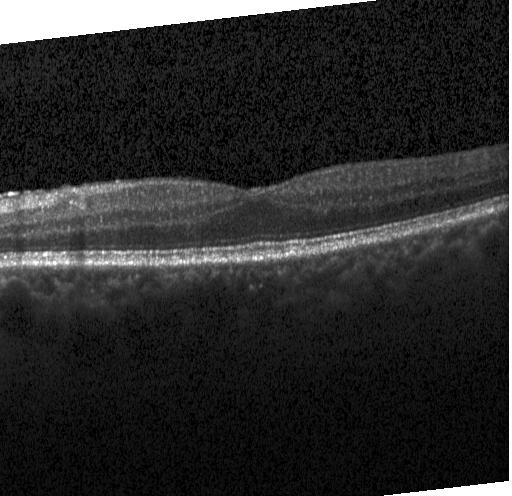 Diagnosis: no CNV, DME, or drusen.